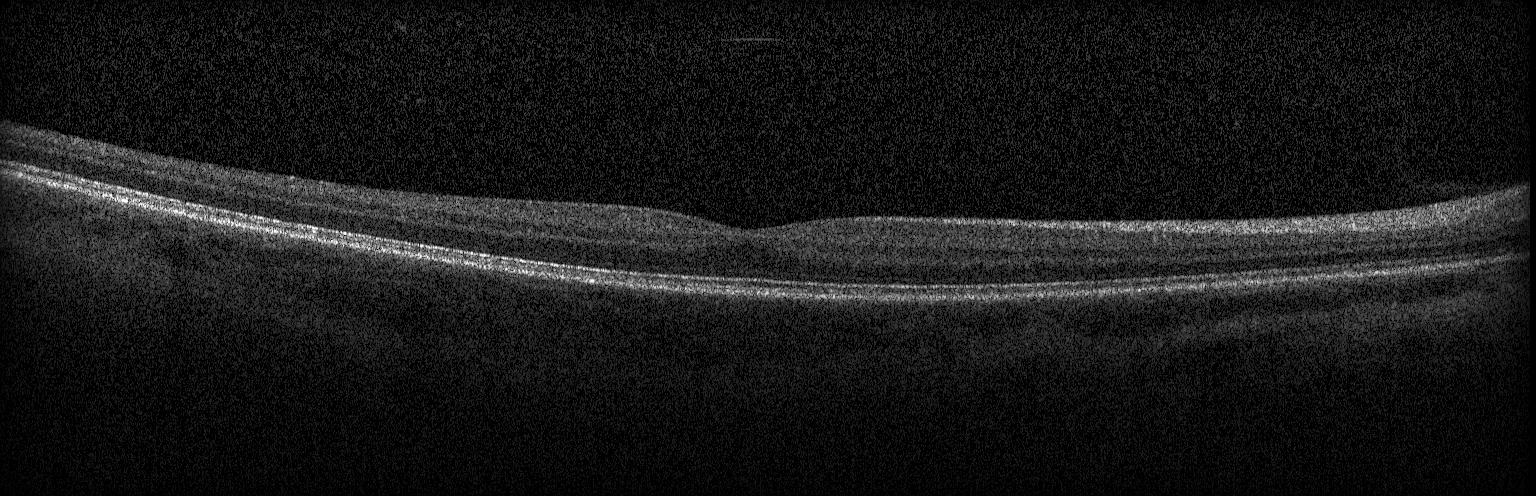

Retinal OCT cross-section
Diagnosis: no evidence of choroidal neovascularization, diabetic macular edema, or drusen.